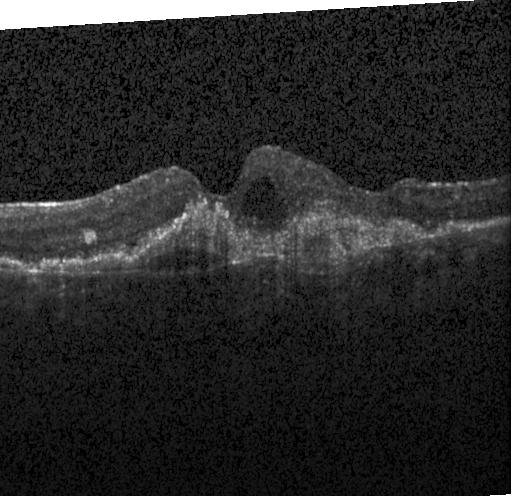 Optical coherence tomography scan — OCT finding: choroidal neovascularization (CNV).